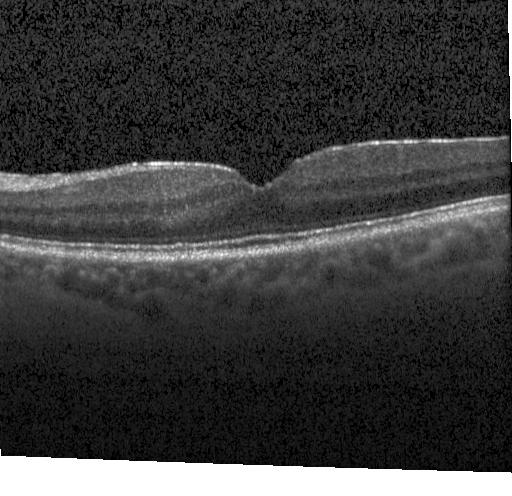

Heidelberg Spectralis OCT system. Spectral-domain OCT. Optical coherence tomography scan. Centered on the fovea
No CNV, DME, or drusen.